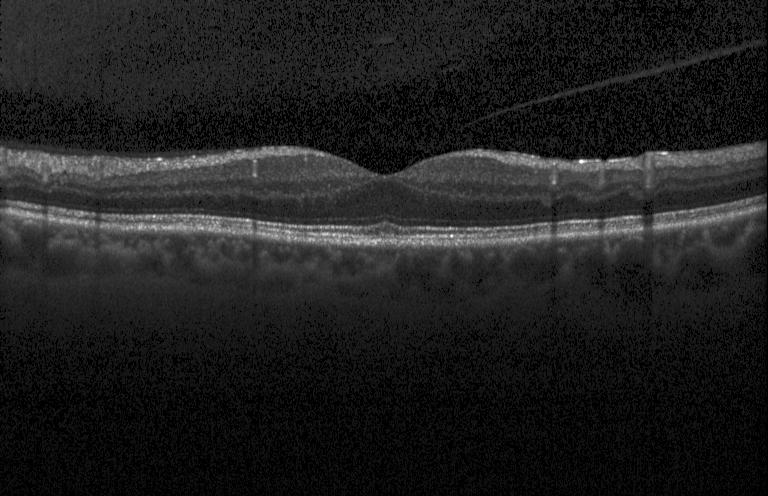 Impression: no evidence of CNV, DME, or drusen.